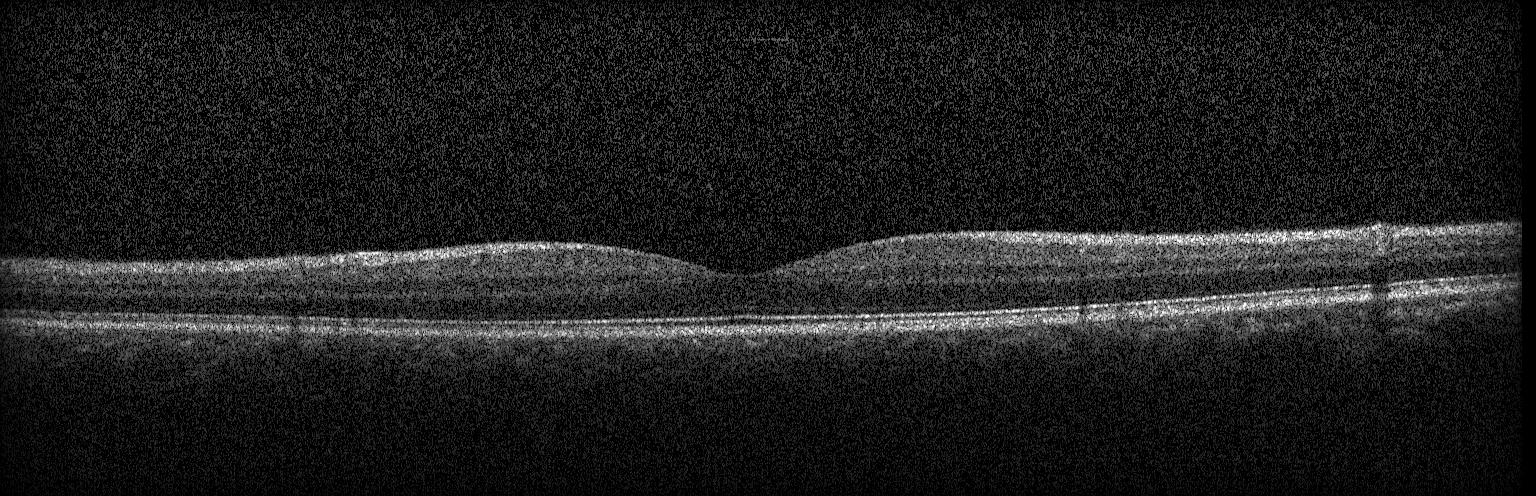

This B-scan demonstrates no evidence of choroidal neovascularization, diabetic macular edema, or drusen.